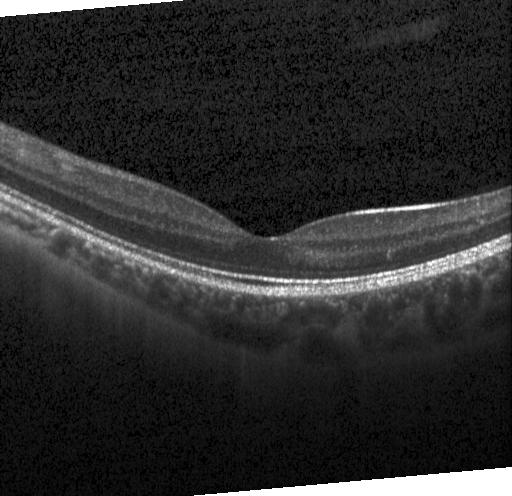
Diagnosis: neither CNV, DME, nor drusen.